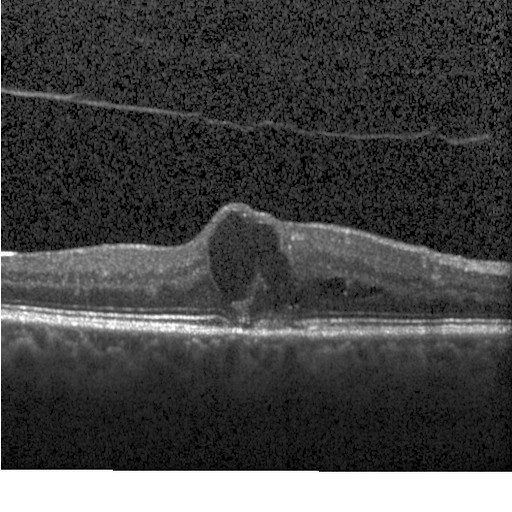
Centered on the fovea; optical coherence tomography B-scan
Diagnosis: diabetic macular edema.